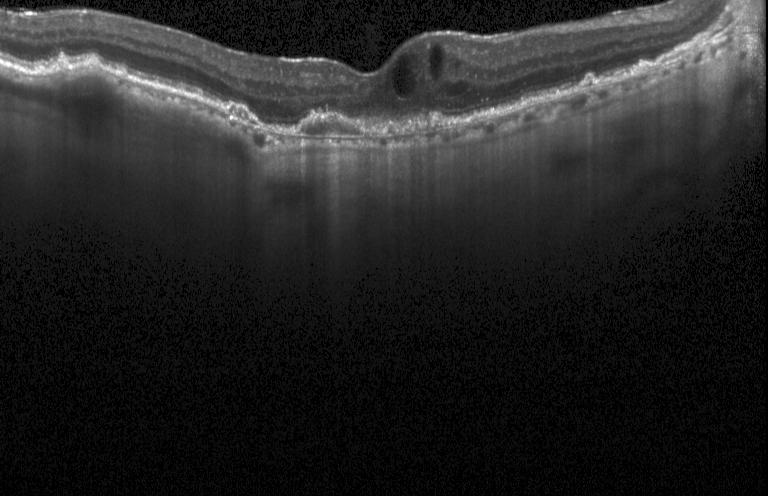 SD-OCT; retinal OCT B-scan — This B-scan demonstrates choroidal neovascularization.